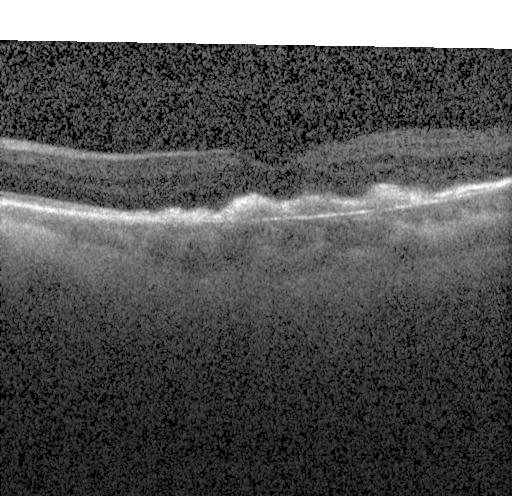 Dx: a choroidal neovascular membrane.